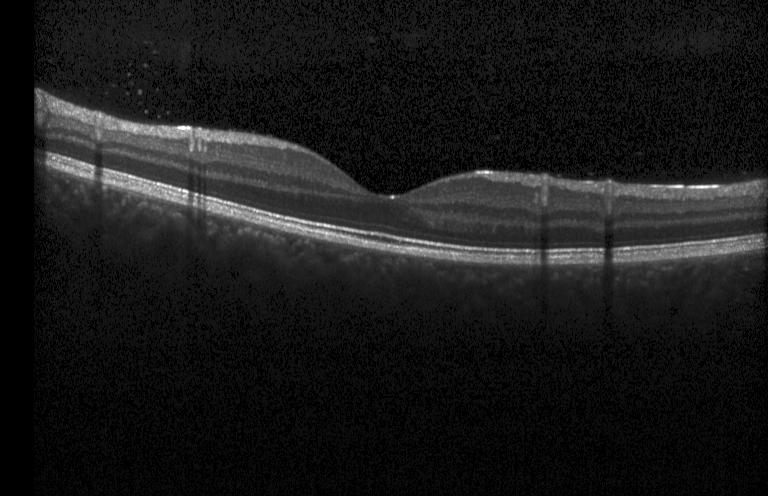 Optical coherence tomography scan, spectral-domain optical coherence tomography. This B-scan demonstrates neither choroidal neovascularization, diabetic macular edema, nor drusen.